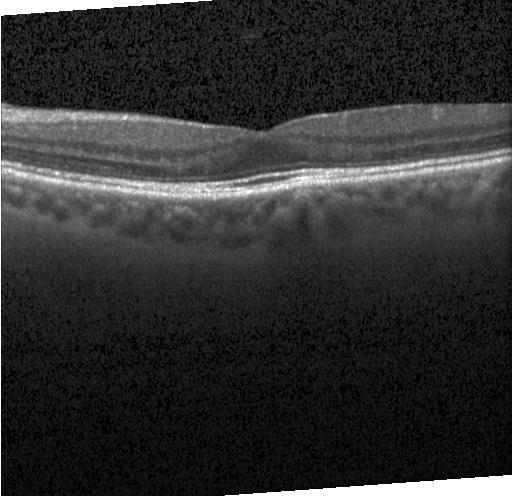
Spectral-domain OCT B-scan: no CNV, DME, or drusen.